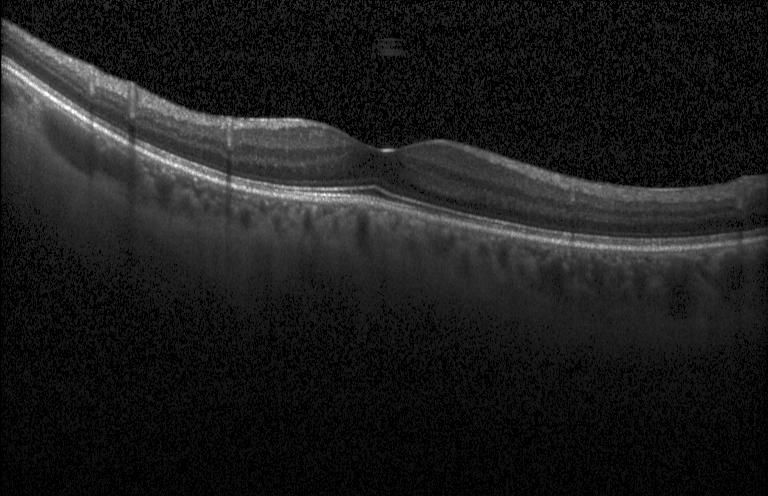
Retinal OCT B-scan
The scan shows no evidence of choroidal neovascularization, diabetic macular edema, or drusen.